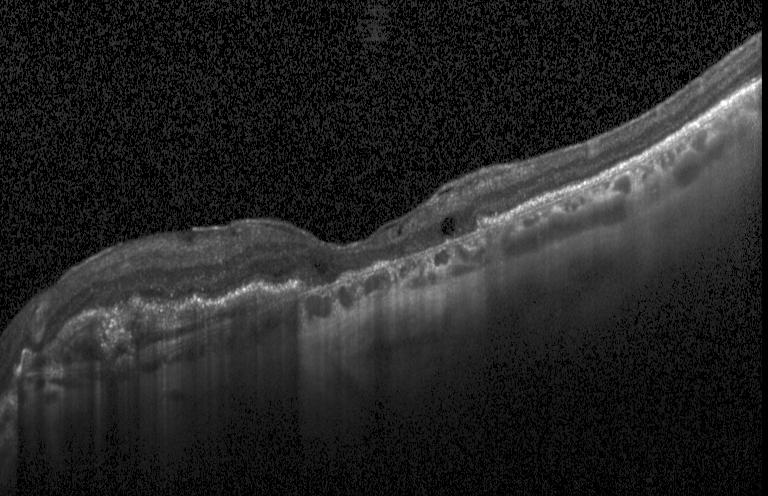
Optical coherence tomography scan — Finding: choroidal neovascularization.